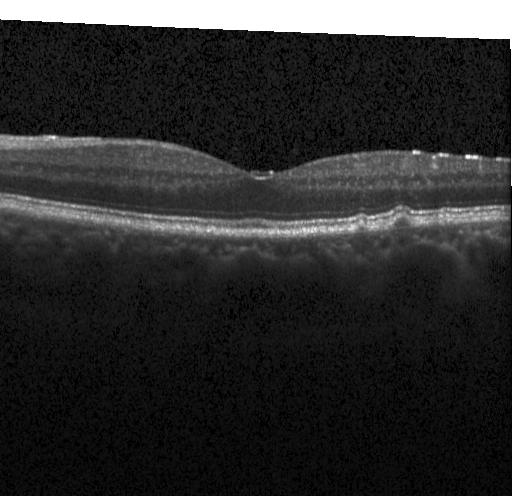

Spectral-domain optical coherence tomography · optical coherence tomography B-scan — Impression: sub-RPE drusenoid deposits.